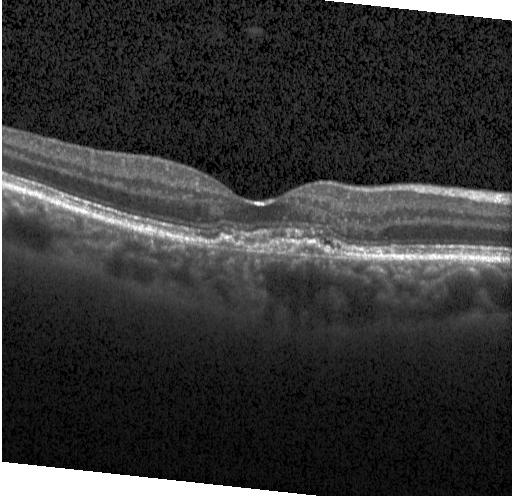
This B-scan demonstrates a choroidal neovascular membrane.